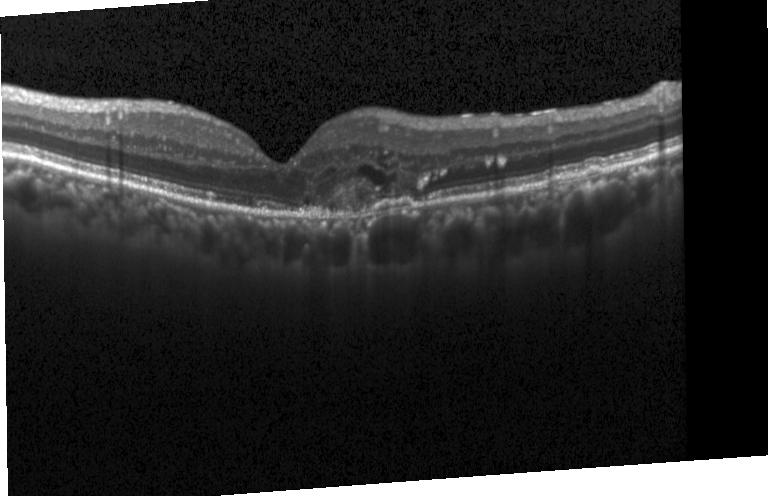 Finding: a choroidal neovascular membrane.